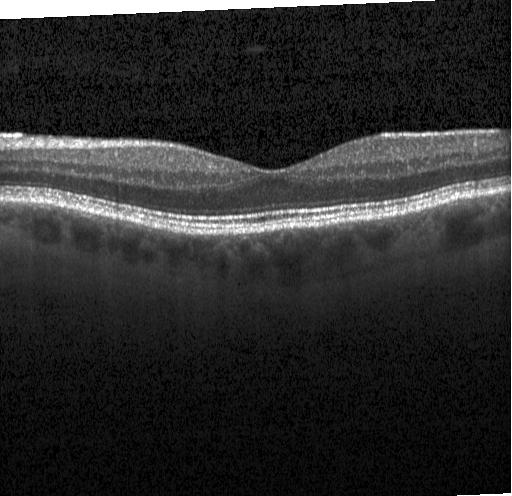 Finding: no choroidal neovascularization, no diabetic macular edema, and no drusen.